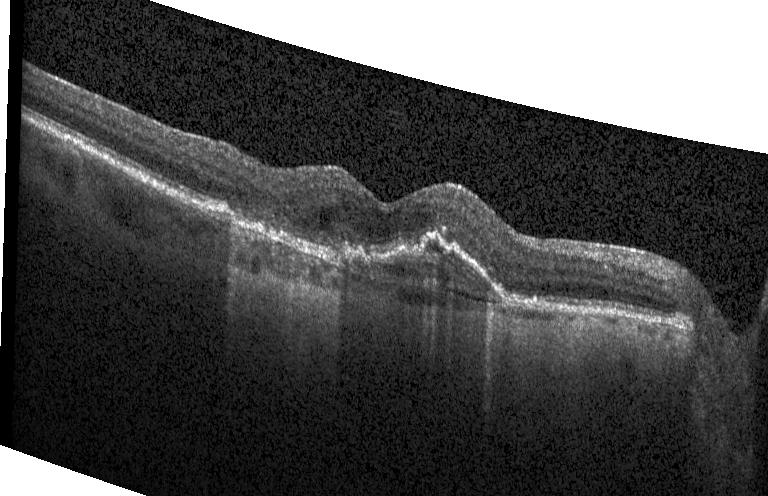

Instrument: Heidelberg Spectralis · OCT line scan · spectral-domain OCT · fovea-centered
Finding: a choroidal neovascular membrane.